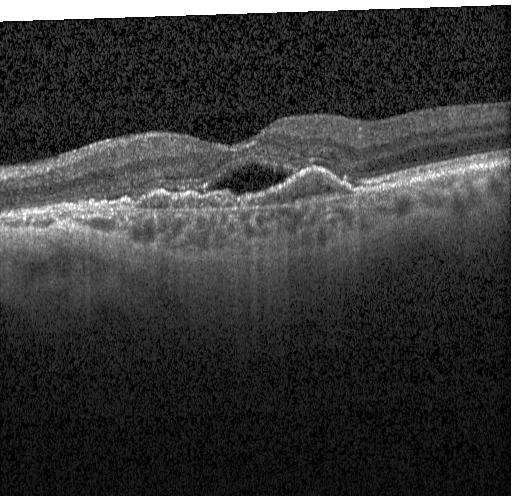

Impression: choroidal neovascularization (CNV).